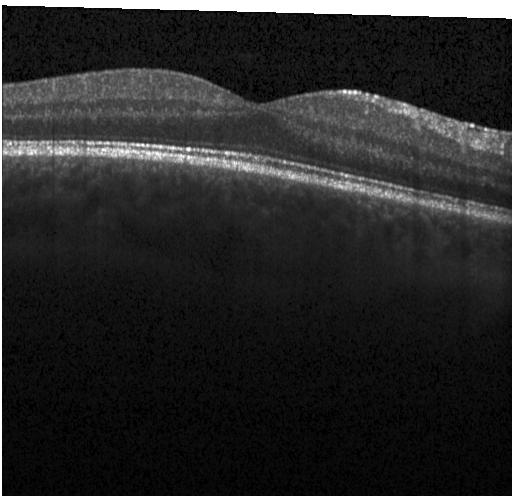

Horizontal scan through the fovea. Optical coherence tomography B-scan. Heidelberg Spectralis OCT system. SD-OCT. No choroidal neovascularization, no diabetic macular edema, and no drusen.